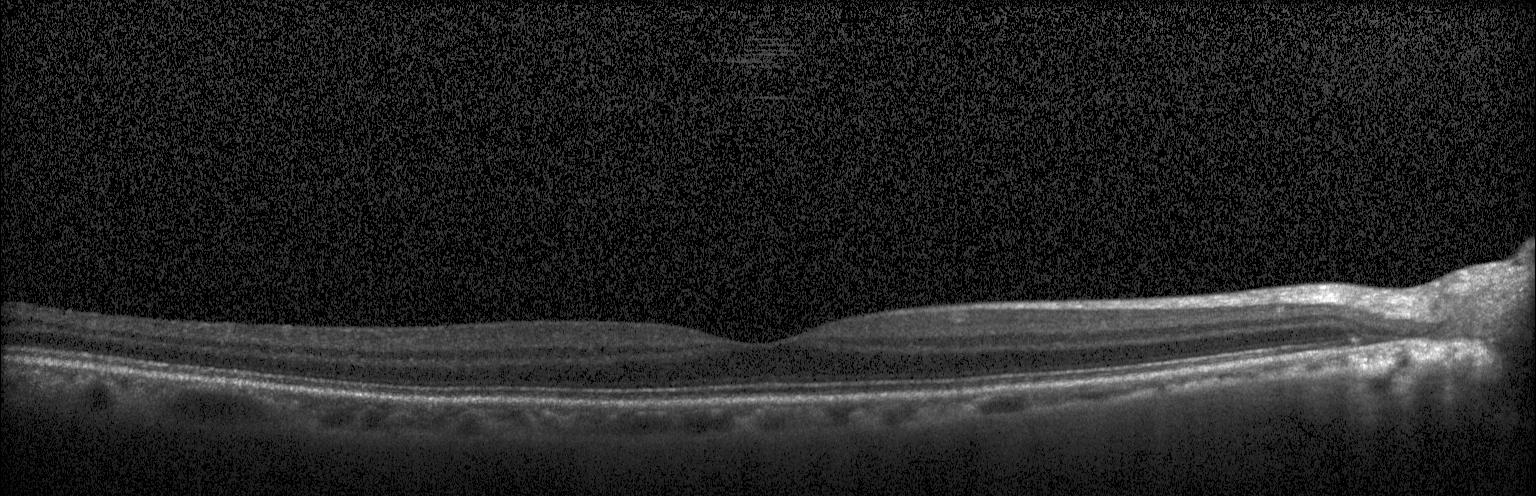
This B-scan demonstrates no choroidal neovascularization, no diabetic macular edema, and no drusen.